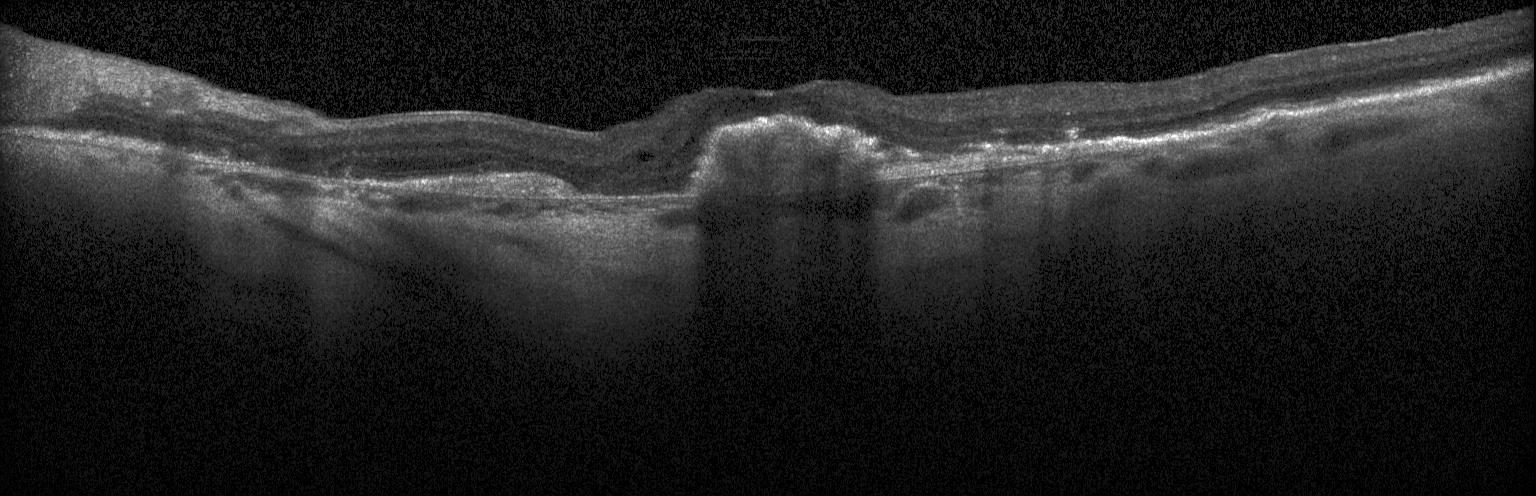 Finding: CNV.